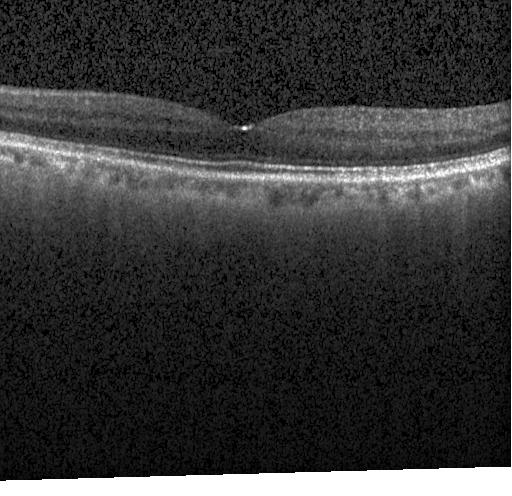

Finding: neither choroidal neovascularization, diabetic macular edema, nor drusen.